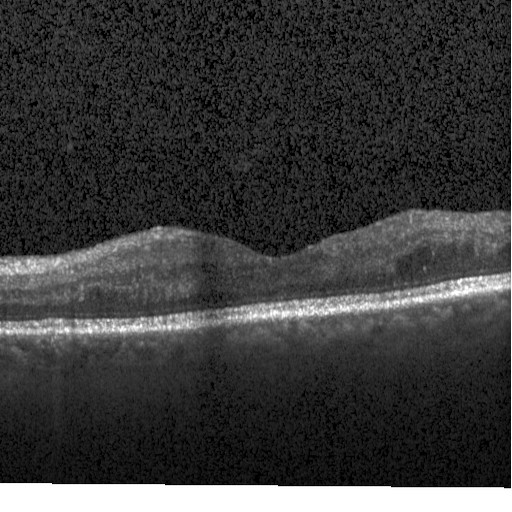 This B-scan demonstrates diabetic macular edema (DME).